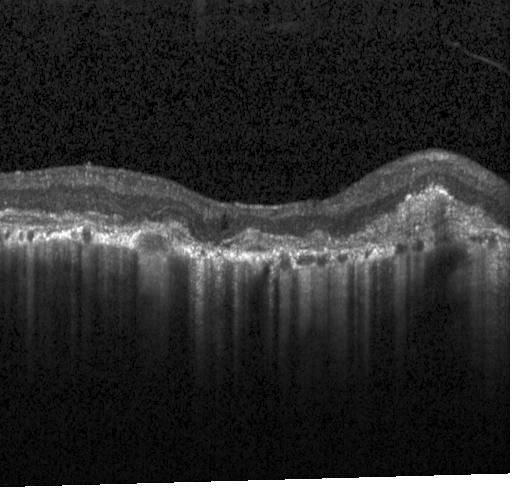
Diagnosis: choroidal neovascularization.